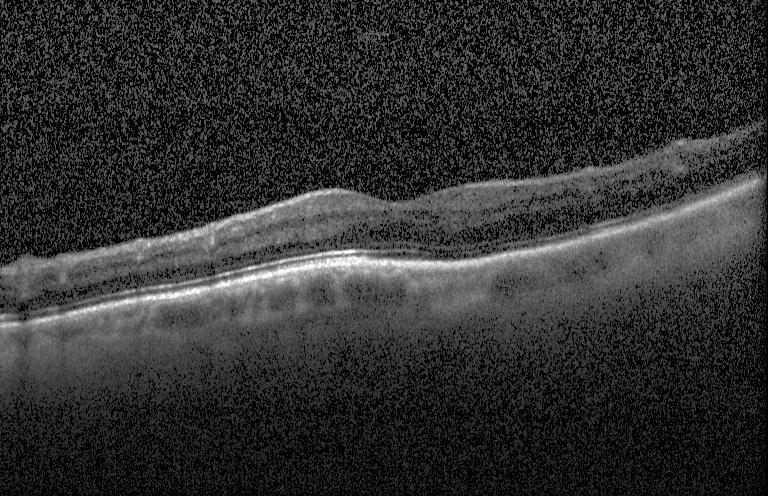

Fovea-centered; SD-OCT; OCT B-scan; Heidelberg Spectralis OCT system.
This B-scan demonstrates no evidence of choroidal neovascularization, diabetic macular edema, or drusen.